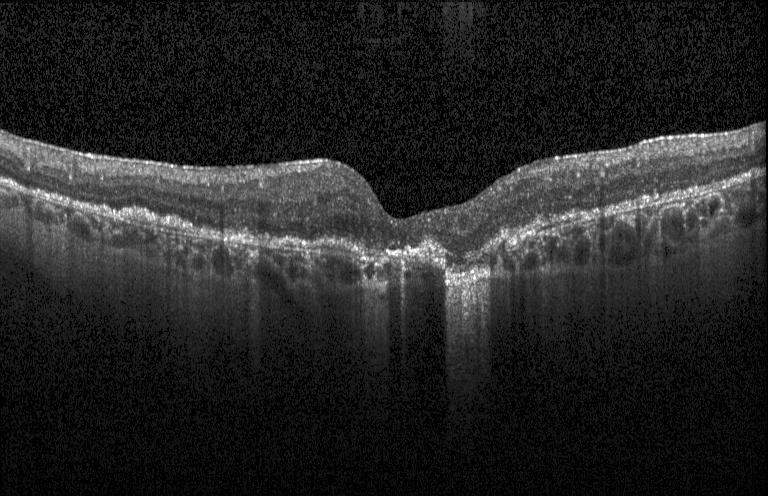 OCT B-scan
A choroidal neovascular membrane.